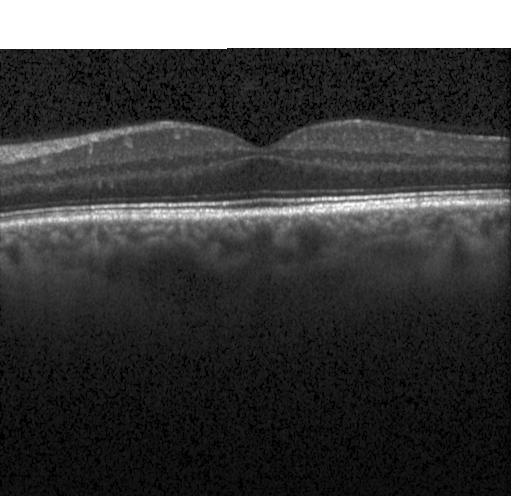 SD-OCT, optical coherence tomography B-scan, horizontal scan through the fovea.
No choroidal neovascularization, diabetic macular edema, or drusen.